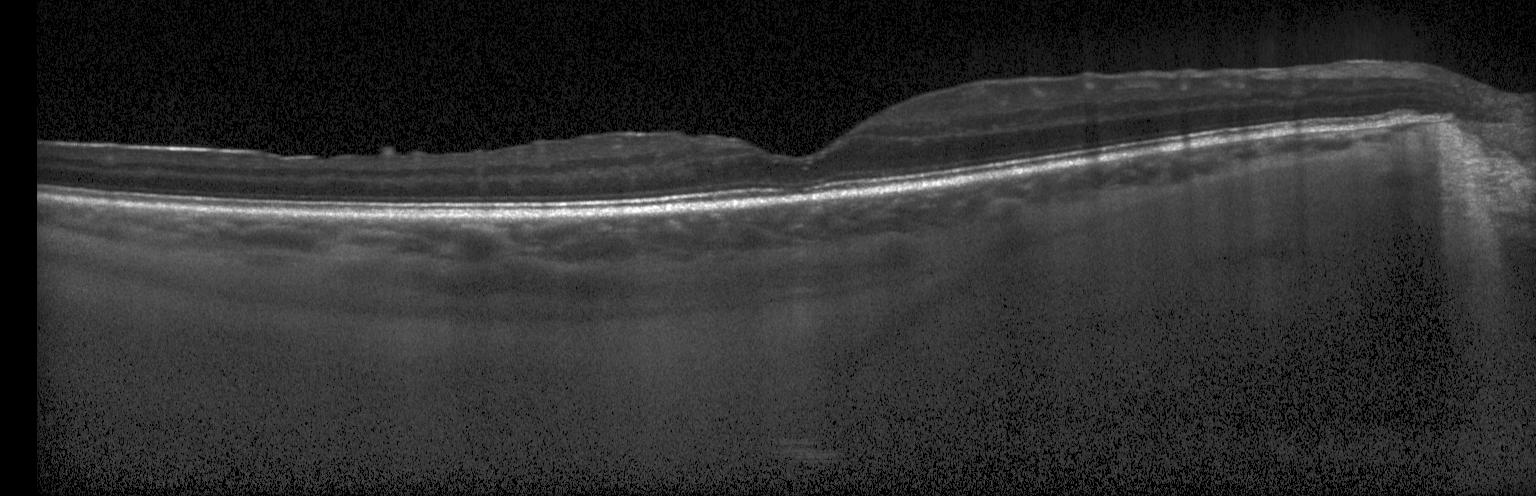
Optical coherence tomography scan — The scan shows no choroidal neovascularization, no diabetic macular edema, and no drusen.